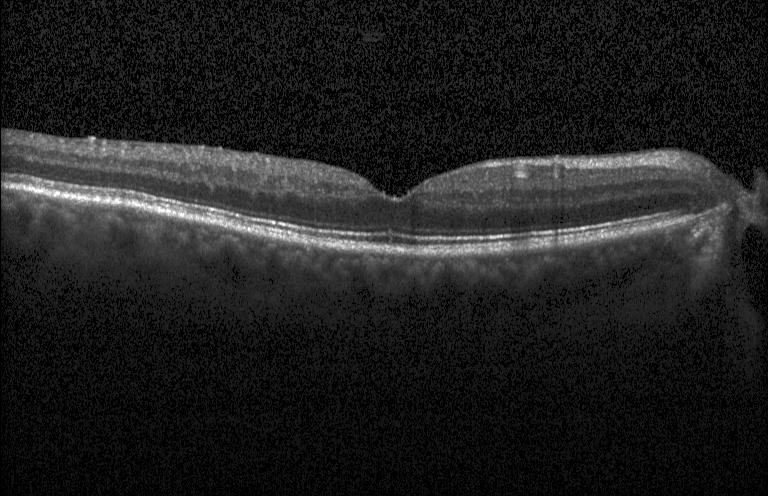

Heidelberg Spectralis, optical coherence tomography scan. This B-scan demonstrates no choroidal neovascularization, diabetic macular edema, or drusen.